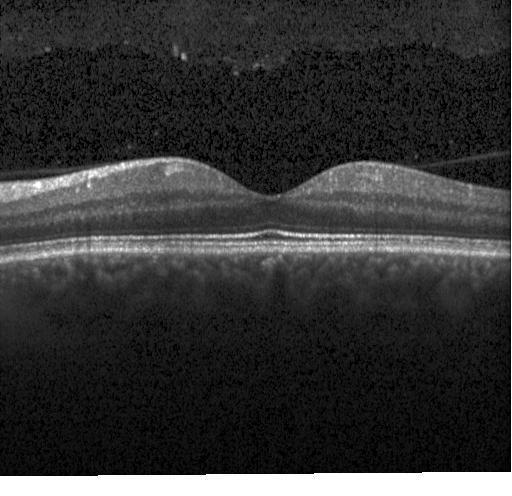
Dx: neither choroidal neovascularization, diabetic macular edema, nor drusen.